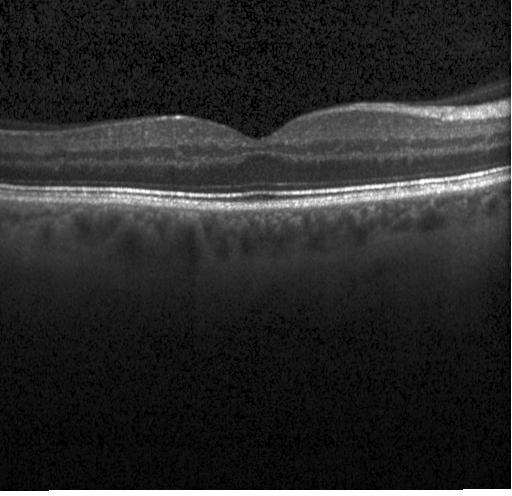

OCT finding: no CNV, DME, or drusen.